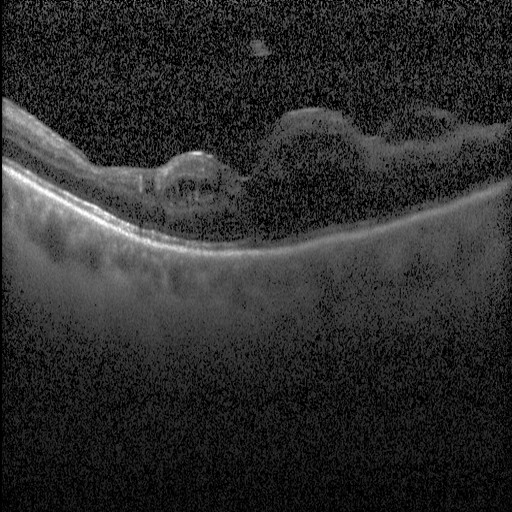

Impression: DME.